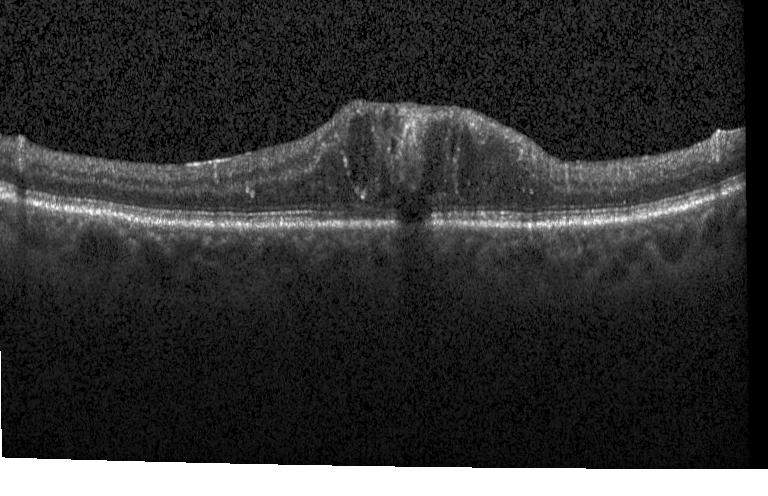
OCT finding: diabetic macular edema (DME).